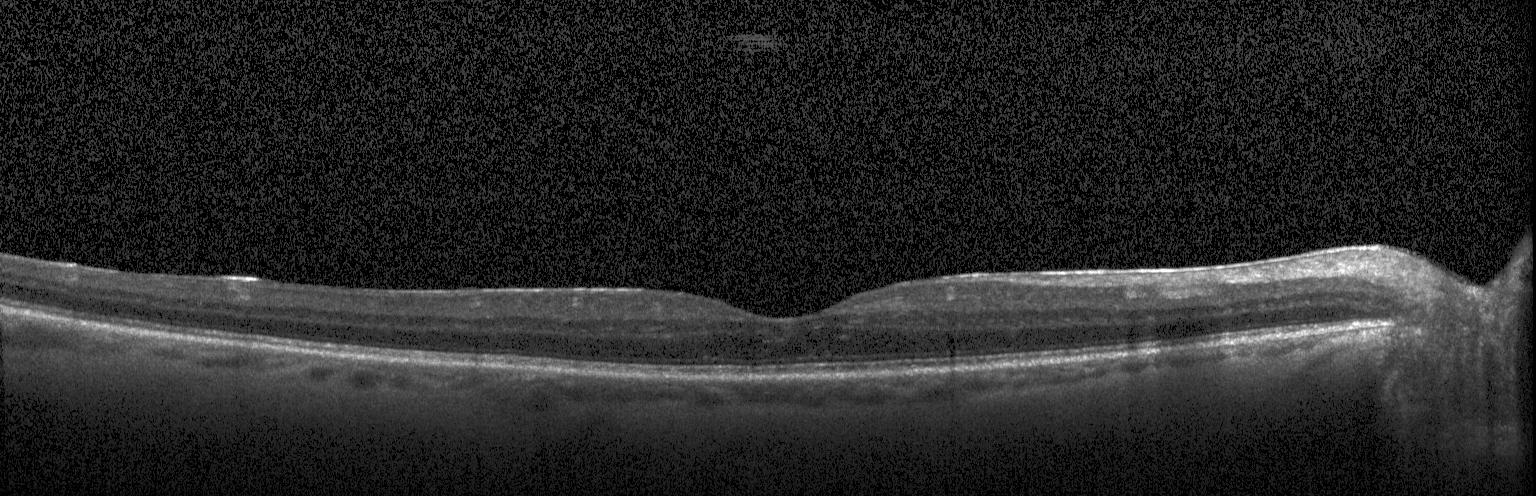

Optical coherence tomography B-scan — Assessment: no choroidal neovascularization, no diabetic macular edema, and no drusen.